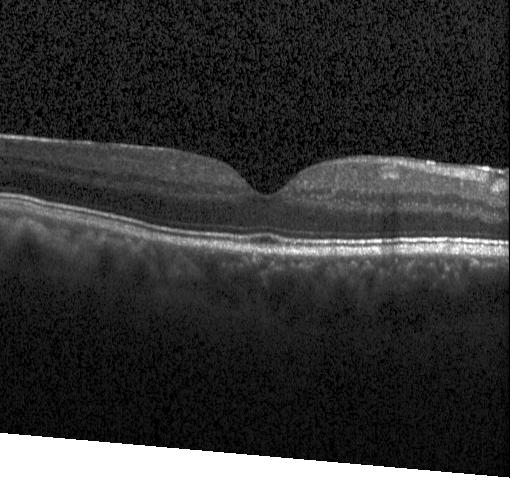 Impression: neither CNV, DME, nor drusen.